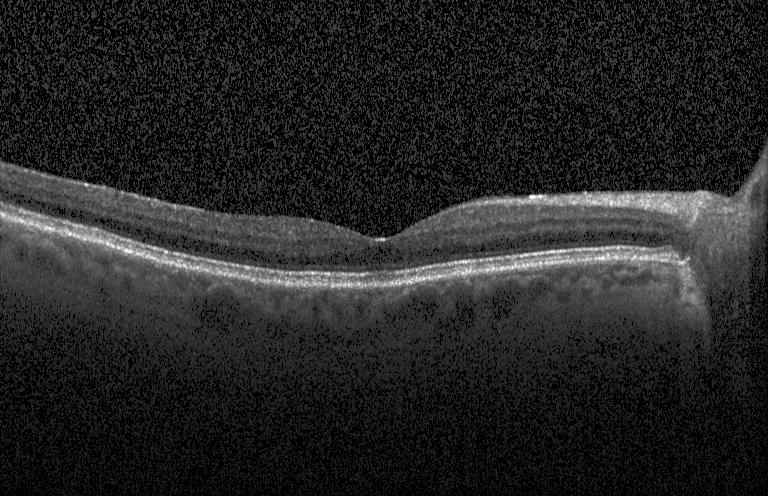 Dx: no choroidal neovascularization, diabetic macular edema, or drusen.